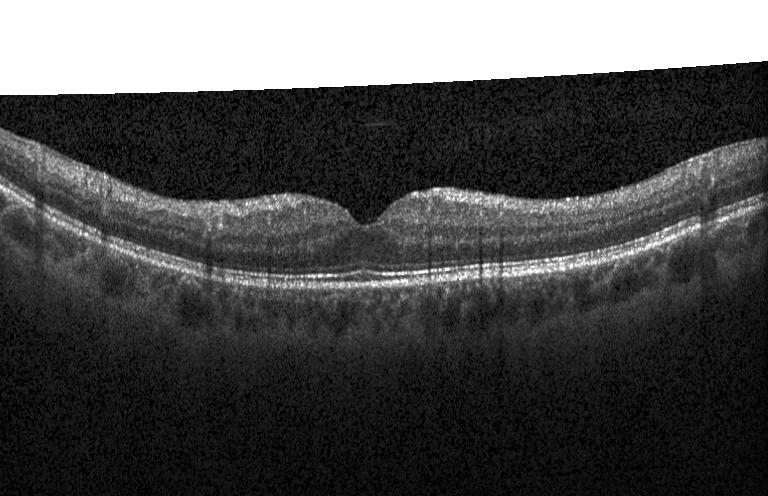
OCT finding: neither CNV, DME, nor drusen.